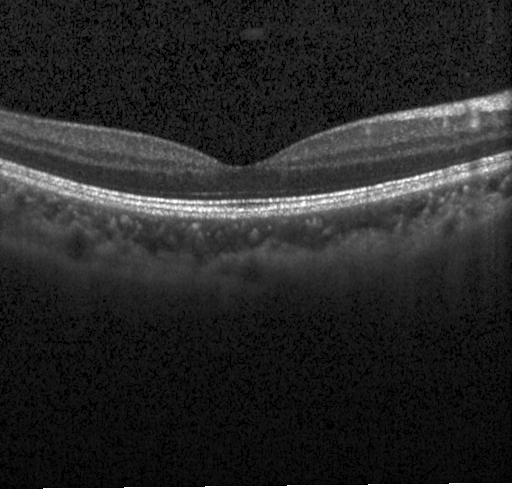 Dx: no CNV, DME, or drusen.